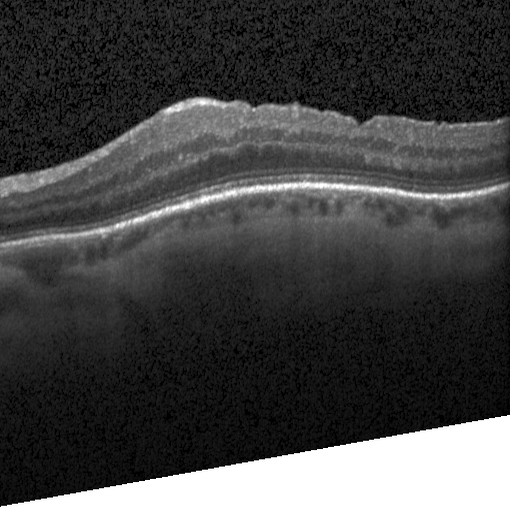 Retinal OCT cross-section, Heidelberg Spectralis OCT system, fovea-centered, spectral-domain optical coherence tomography. Finding: diabetic macular edema.